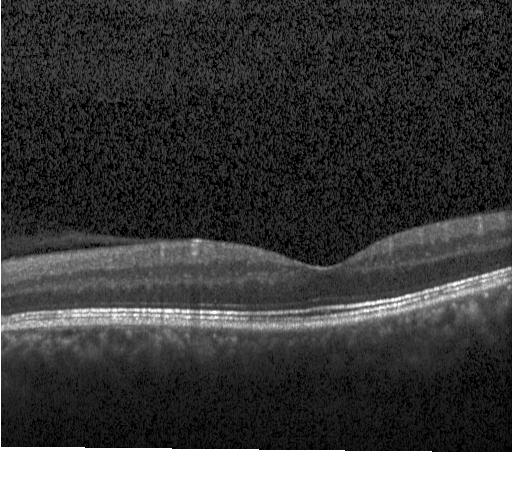
Retinal OCT B-scan — Diagnosis: neither CNV, DME, nor drusen.